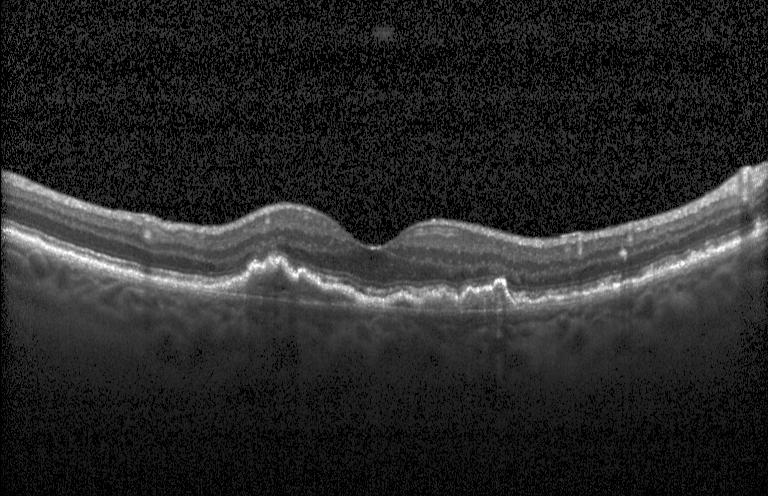 The scan shows a choroidal neovascular membrane.